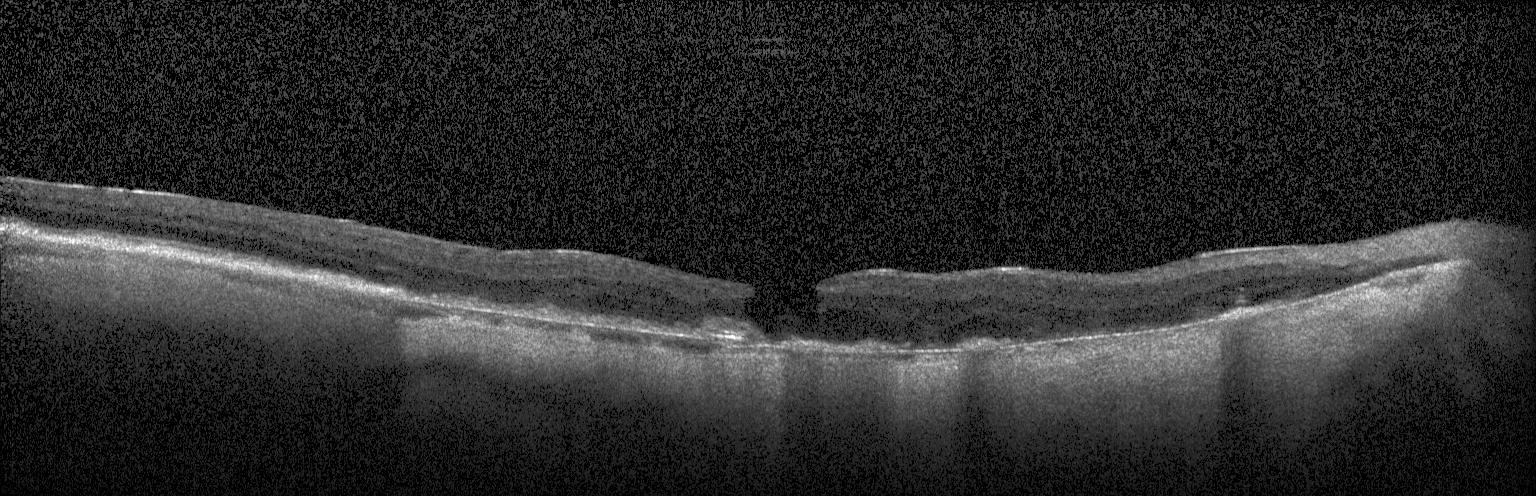

Macular OCT: a choroidal neovascular membrane.